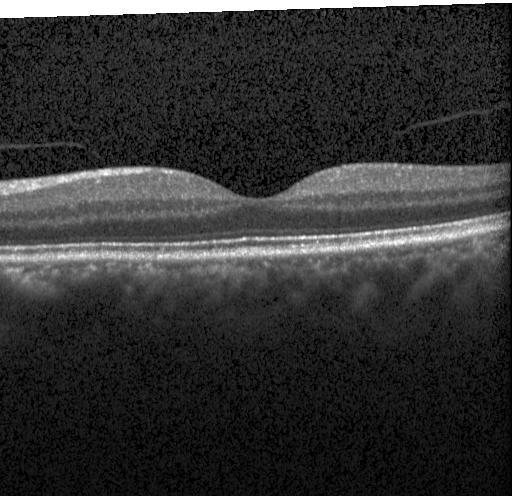 No CNV, no DME, and no drusen.